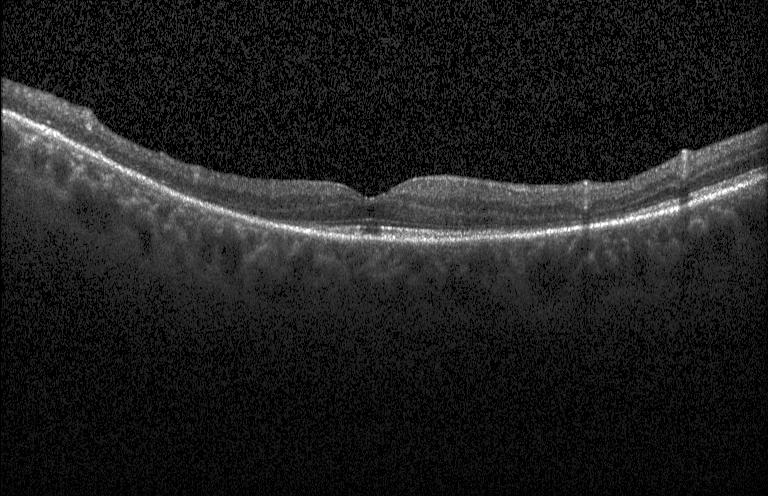
OCT B-scan showing no evidence of choroidal neovascularization, diabetic macular edema, or drusen.